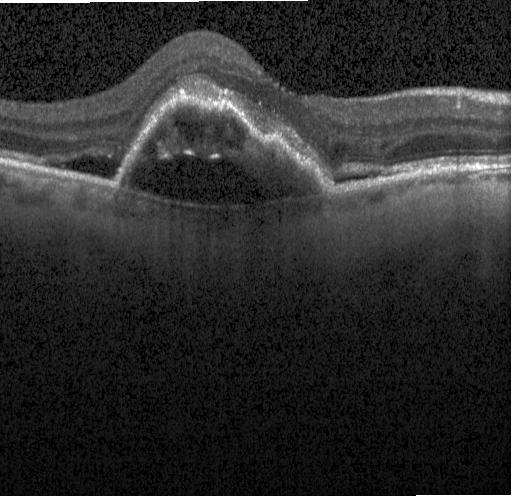

Macular scan · OCT B-scan · acquired on a Heidelberg Spectralis. The scan shows choroidal neovascularization (CNV).